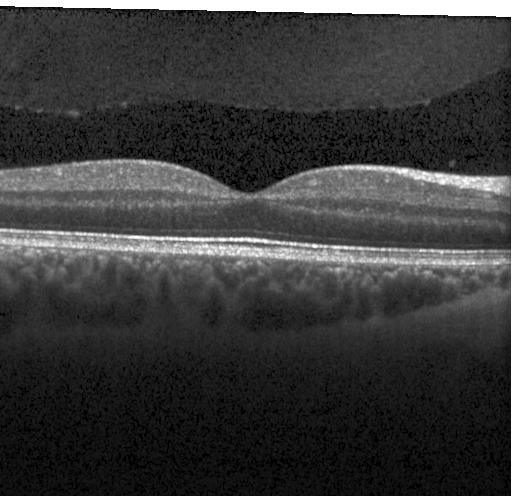 Macular OCT: no evidence of CNV, DME, or drusen.